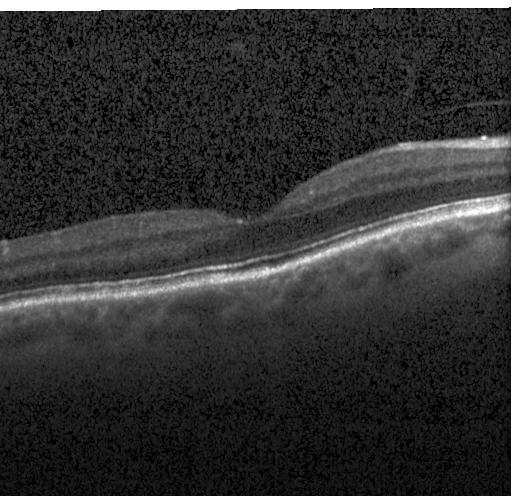 Finding: no evidence of CNV, DME, or drusen.